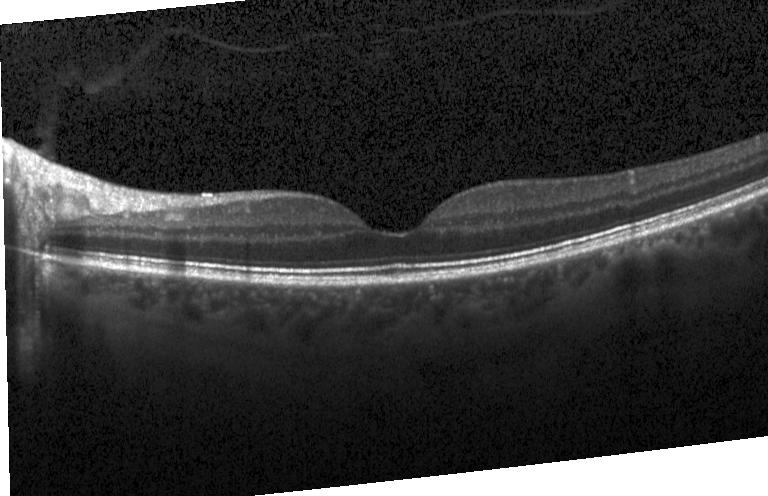
Spectral-domain OCT B-scan: no CNV, DME, or drusen.